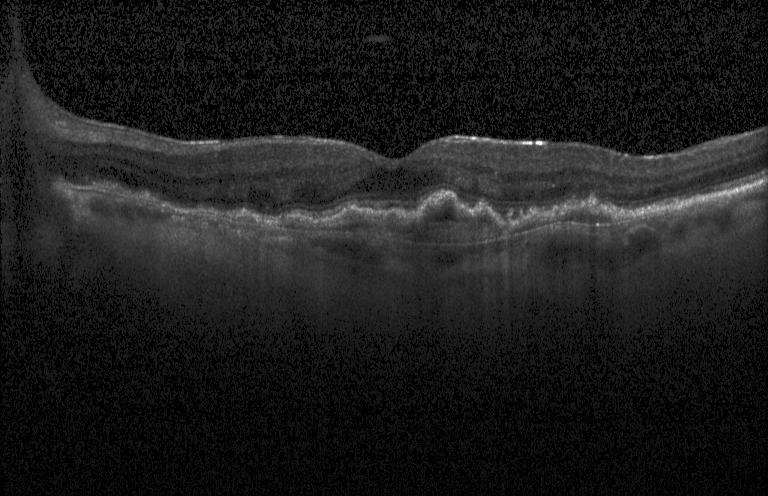
OCT B-scan showing a choroidal neovascular membrane.